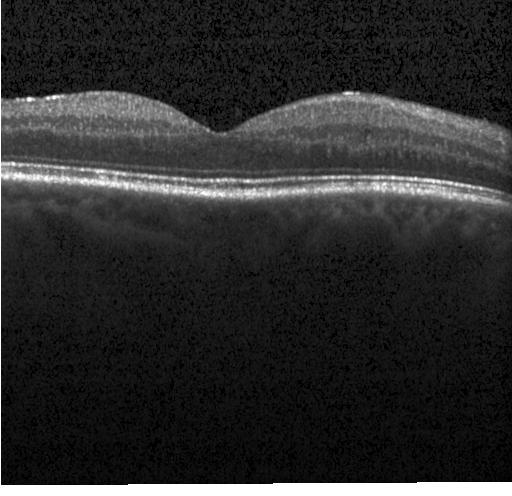
OCT finding: no evidence of choroidal neovascularization, diabetic macular edema, or drusen.